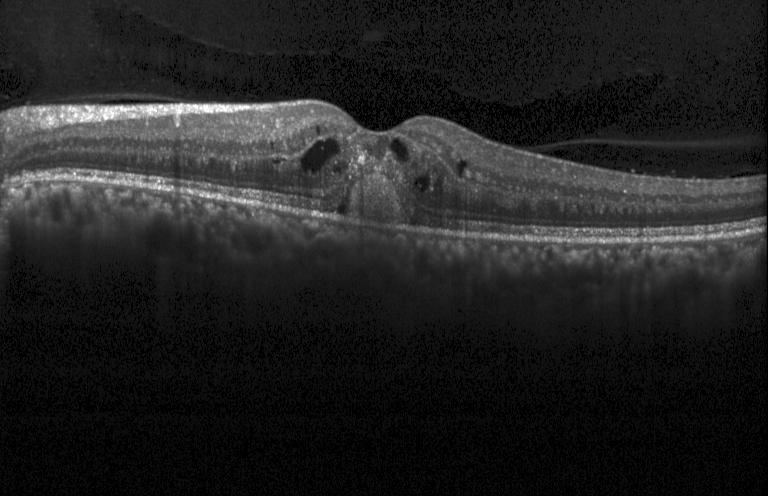
SD-OCT. Optical coherence tomography B-scan. Through the macula
CNV.